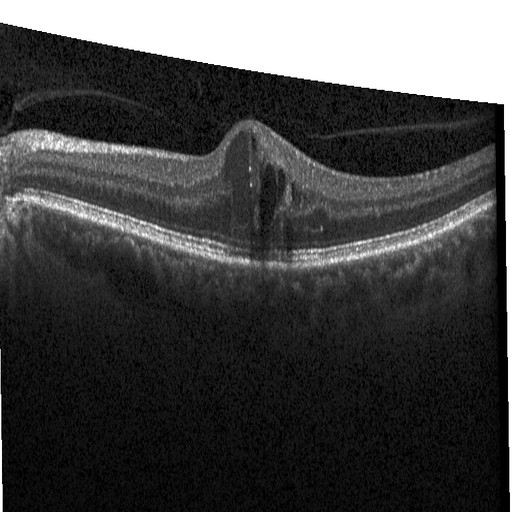

Macular OCT: diabetic macular edema.